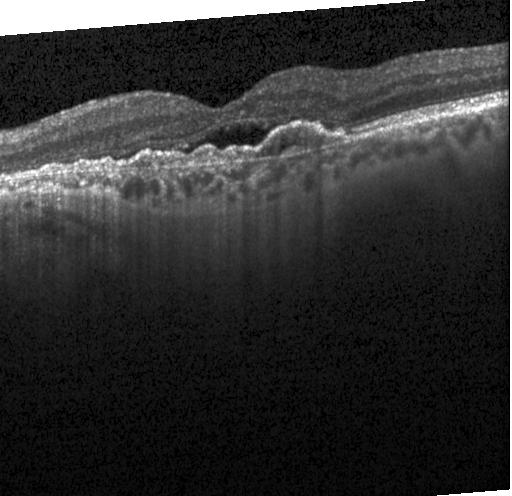 OCT line scan, spectral-domain OCT
Diagnosis: CNV.